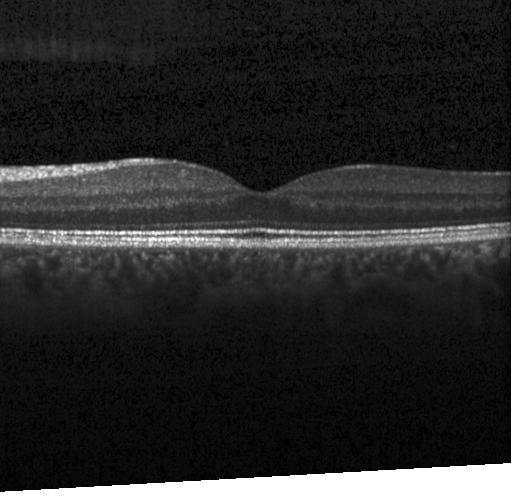

Retinal OCT B-scan
Macular OCT: no CNV, no DME, and no drusen.